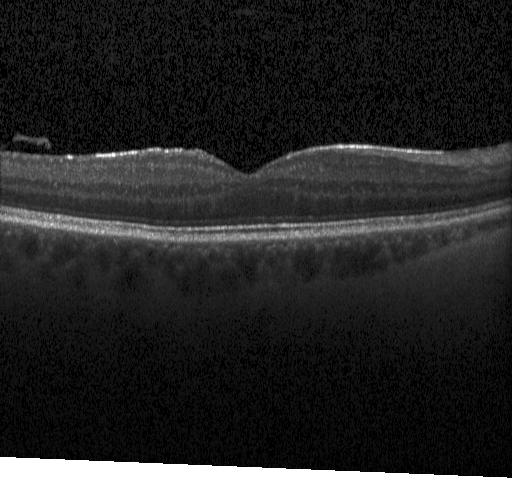
Finding: neither choroidal neovascularization, diabetic macular edema, nor drusen.